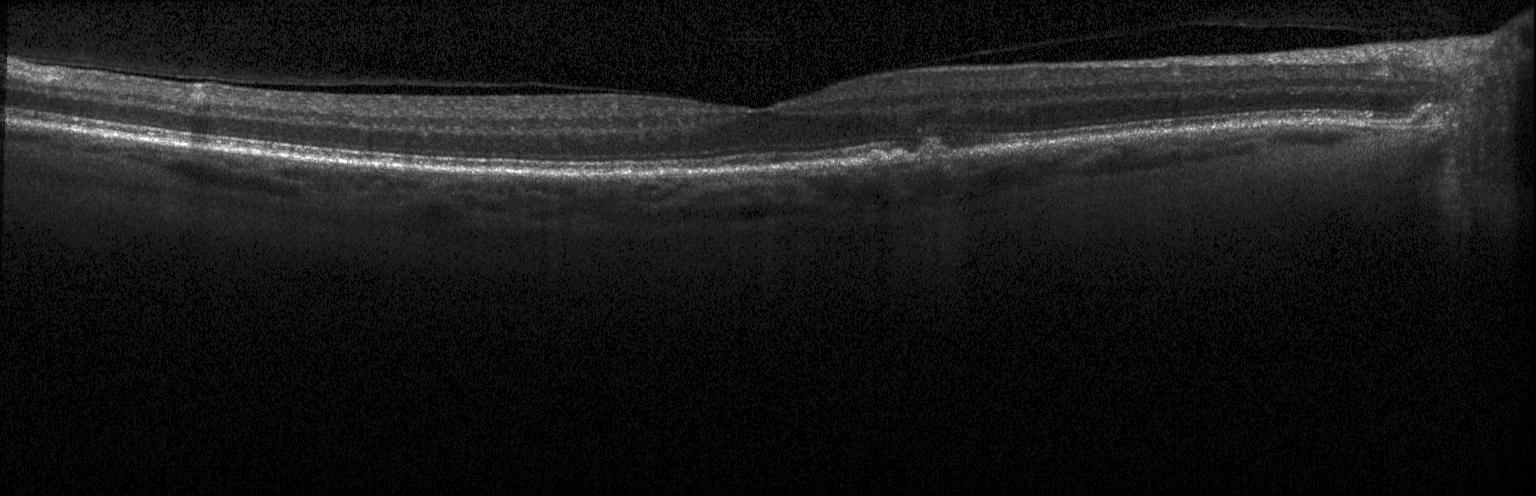
Fovea-centered. OCT line scan. Heidelberg Spectralis OCT system. Spectral-domain OCT.
Drusen.